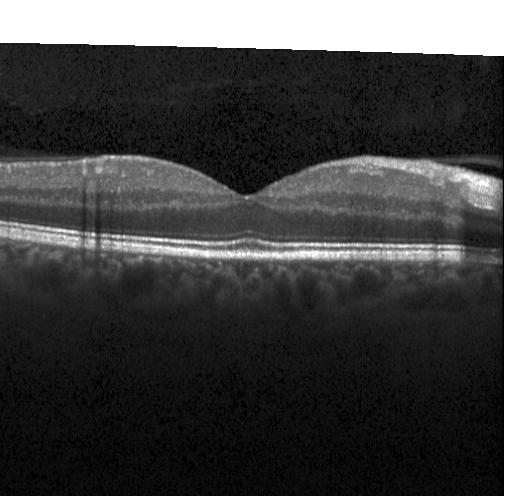
Macular OCT: no CNV, no DME, and no drusen.